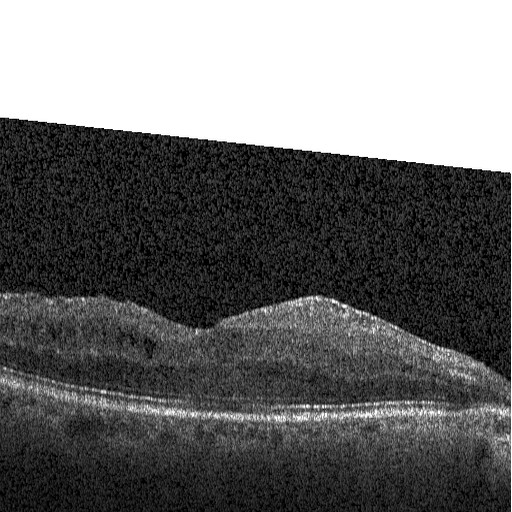

Spectral-domain OCT B-scan: diabetic macular edema.